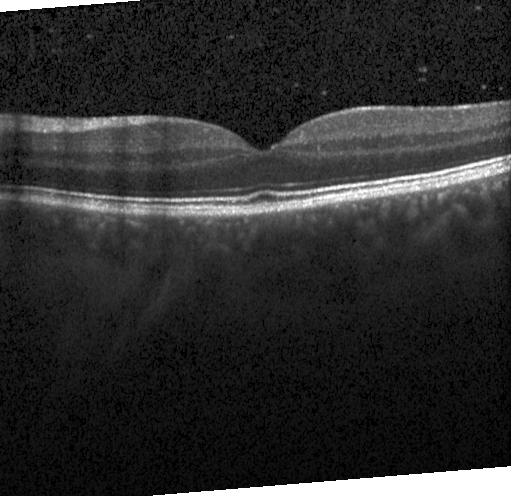
Dx: no CNV, no DME, and no drusen.